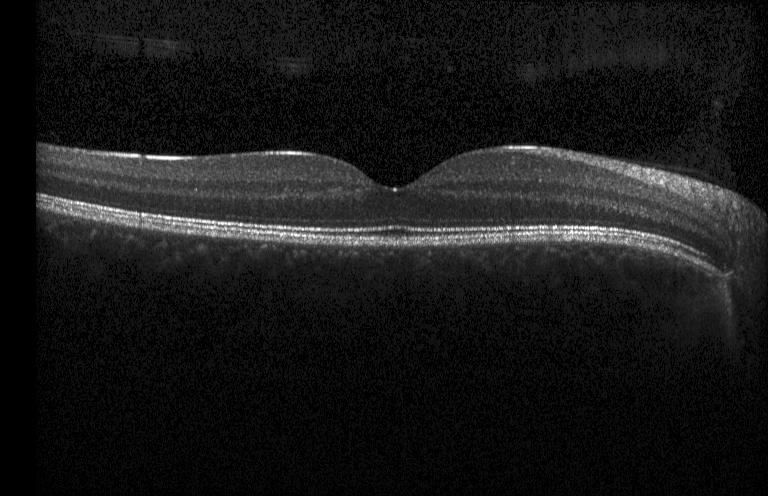

Assessment: no evidence of choroidal neovascularization, diabetic macular edema, or drusen.